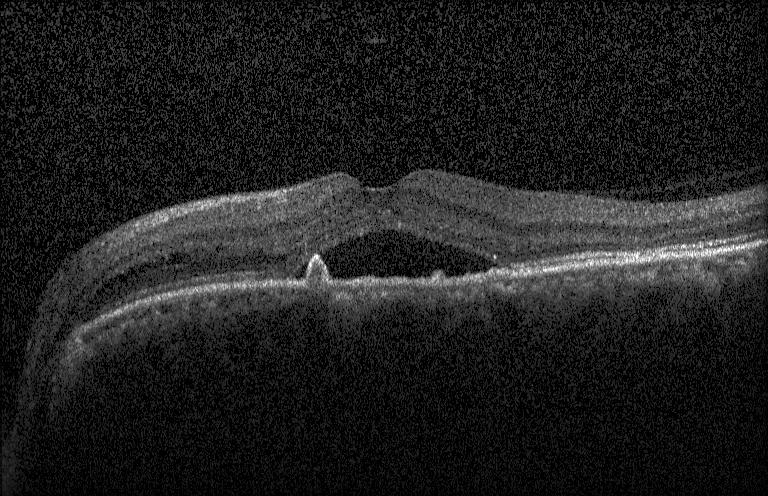
Optical coherence tomography B-scan.
Finding: a choroidal neovascular membrane.